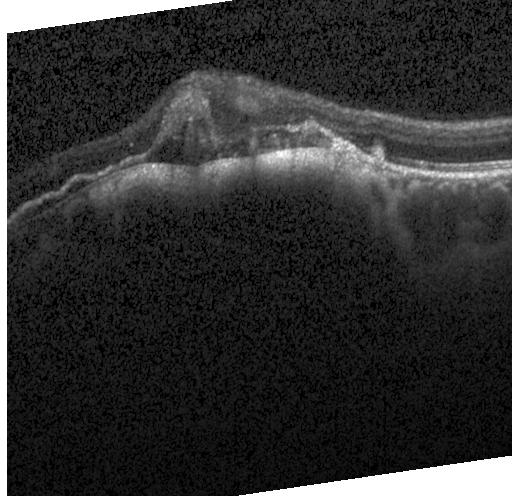
Centered on the fovea, retinal OCT cross-section.
Assessment: CNV.